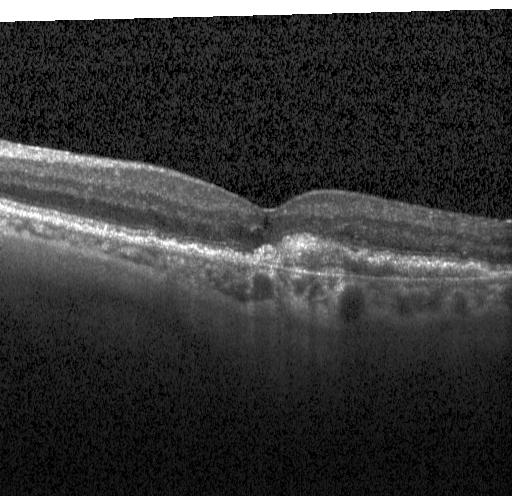
Spectral-domain OCT B-scan: a choroidal neovascular membrane.